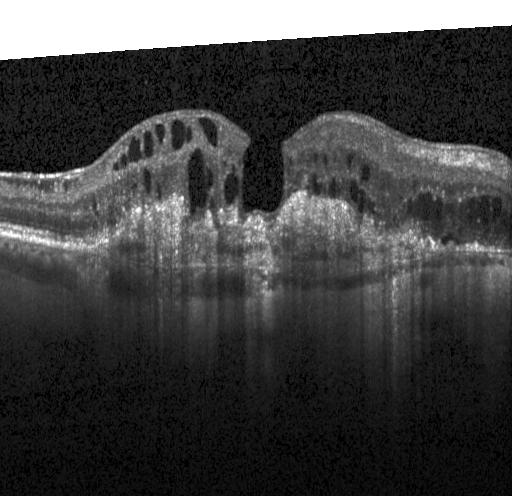
Dx: choroidal neovascularization (CNV).